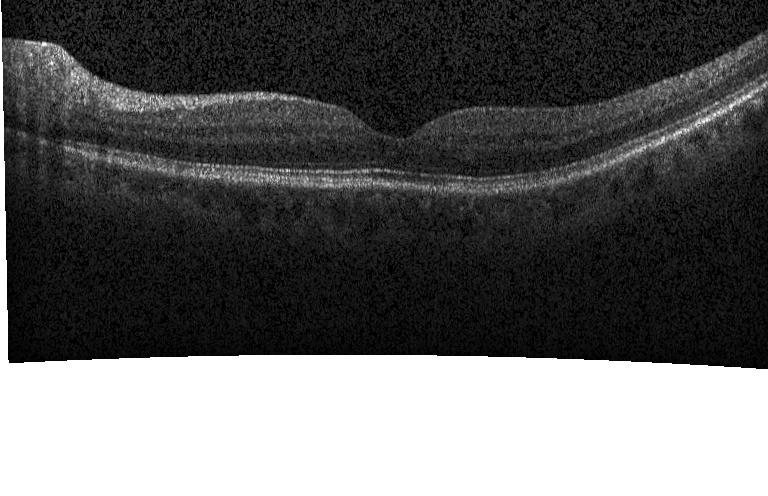

Retinal OCT cross-section; Heidelberg Spectralis — OCT finding: neither CNV, DME, nor drusen.